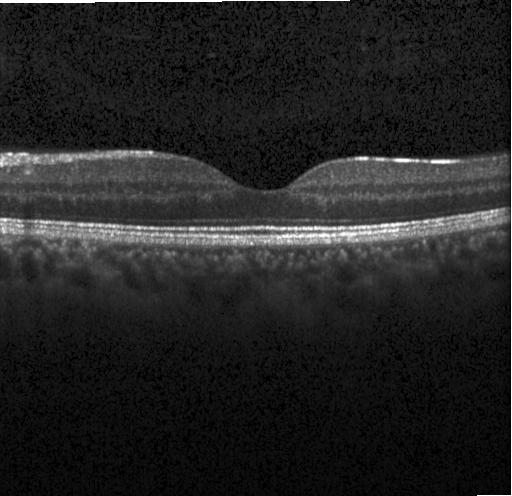 Heidelberg Spectralis · OCT line scan — The scan shows neither CNV, DME, nor drusen.